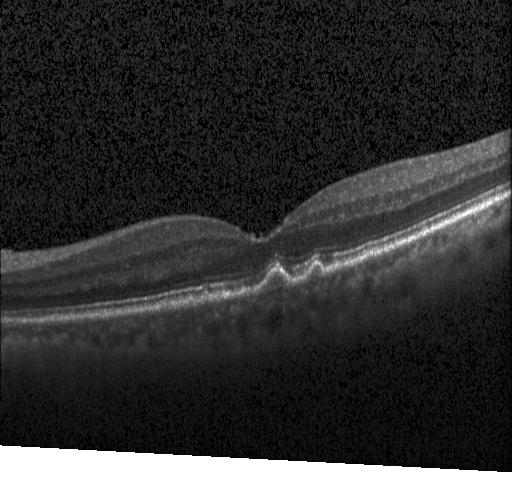

Retinal OCT cross-section; centered on the fovea; spectral-domain optical coherence tomography; Heidelberg Spectralis — Dx: drusen.